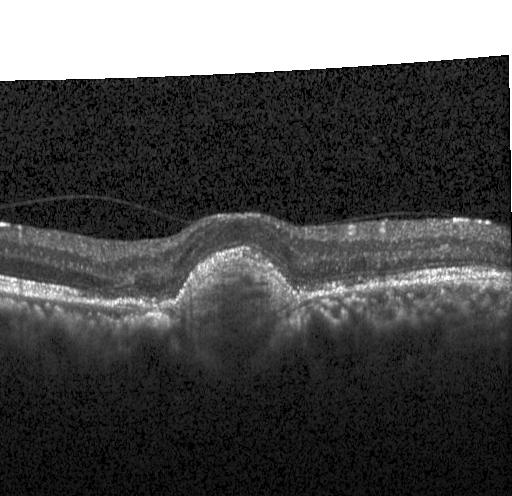
Retinal OCT B-scan. Spectral-domain optical coherence tomography — Finding: a choroidal neovascular membrane.